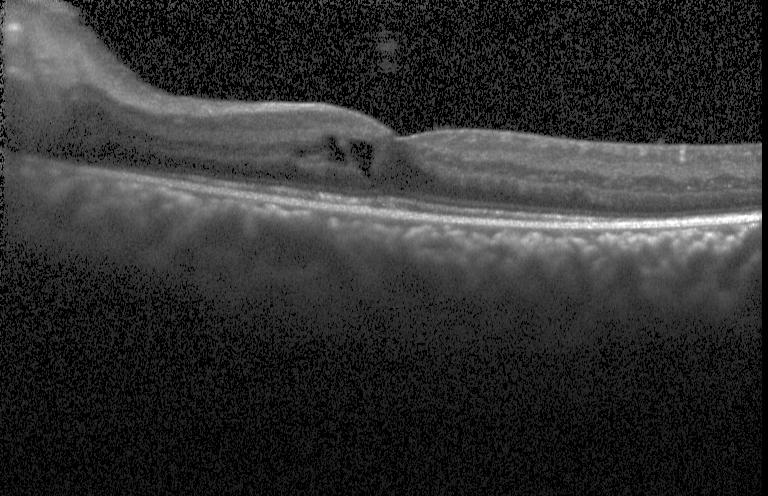 Macular scan. OCT line scan. Instrument: Heidelberg Spectralis.
The scan shows diabetic macular edema (DME).